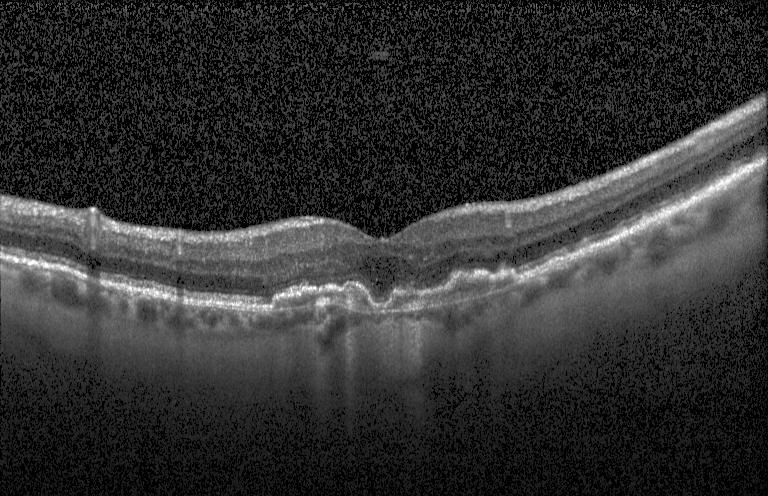

Instrument: Heidelberg Spectralis; optical coherence tomography scan.
Impression: a choroidal neovascular membrane.